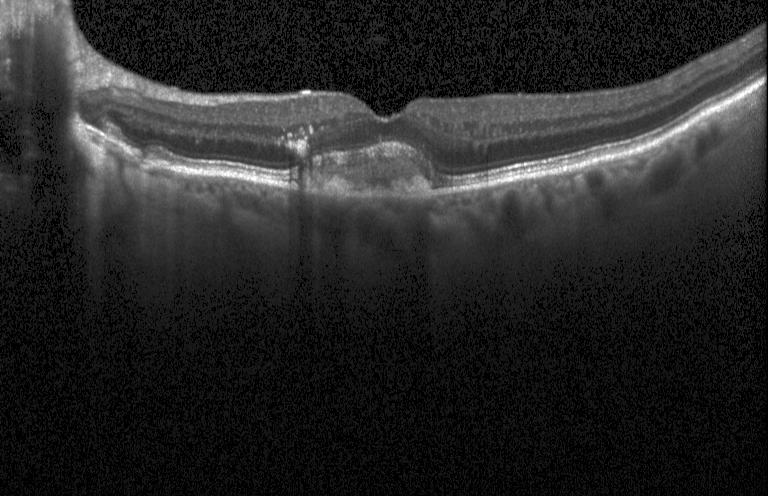

Retinal OCT B-scan. Assessment: CNV.